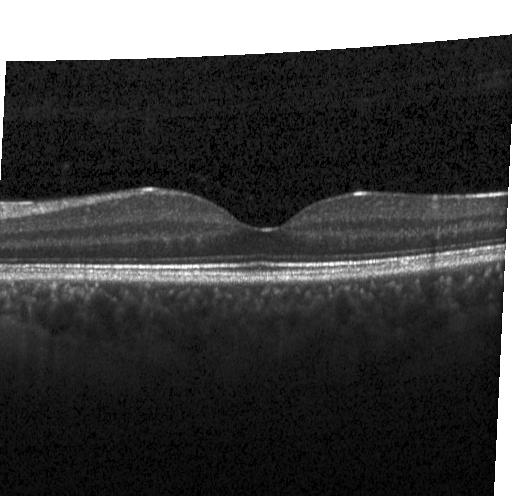 Macular scan. Spectral-domain optical coherence tomography. Retinal OCT cross-section. Macular OCT: neither CNV, DME, nor drusen.